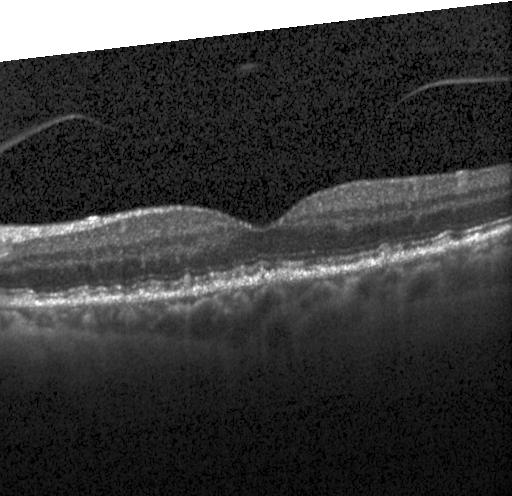
Optical coherence tomography B-scan.
Impression: multiple drusen.